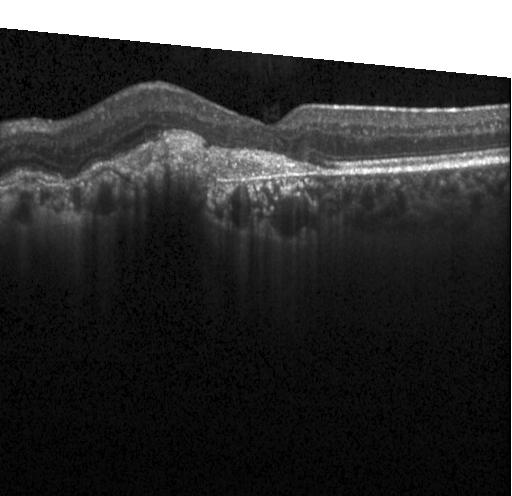

OCT line scan · horizontal scan through the fovea · instrument: Heidelberg Spectralis · spectral-domain OCT — Diagnosis: a choroidal neovascular membrane.